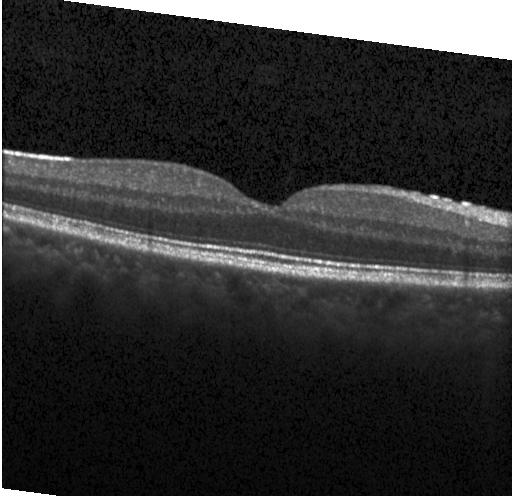 Retinal OCT cross-section. Dx: no choroidal neovascularization, no diabetic macular edema, and no drusen.